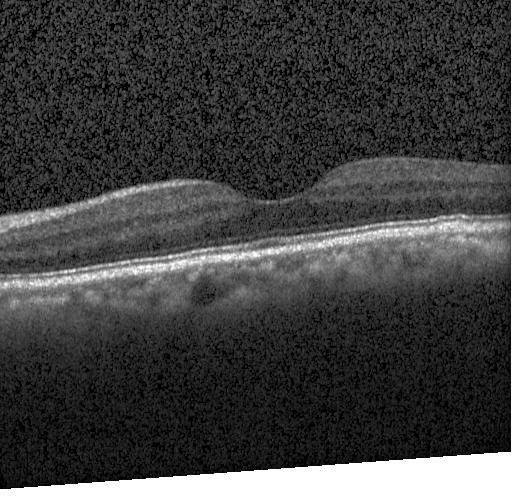 OCT line scan. Through the macula.
Impression: no evidence of choroidal neovascularization, diabetic macular edema, or drusen.